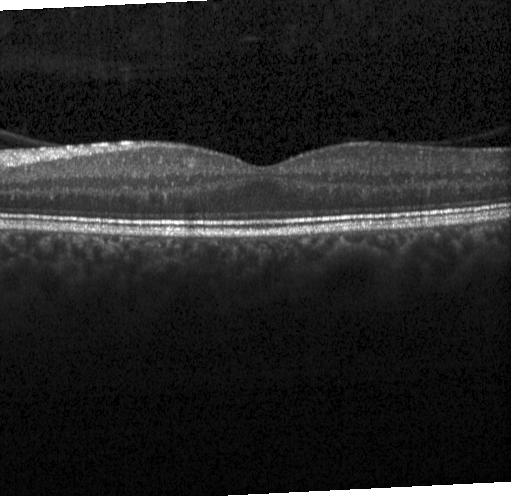
Spectral-domain optical coherence tomography, Heidelberg Spectralis, centered on the fovea, optical coherence tomography B-scan — Impression: no CNV, no DME, and no drusen.